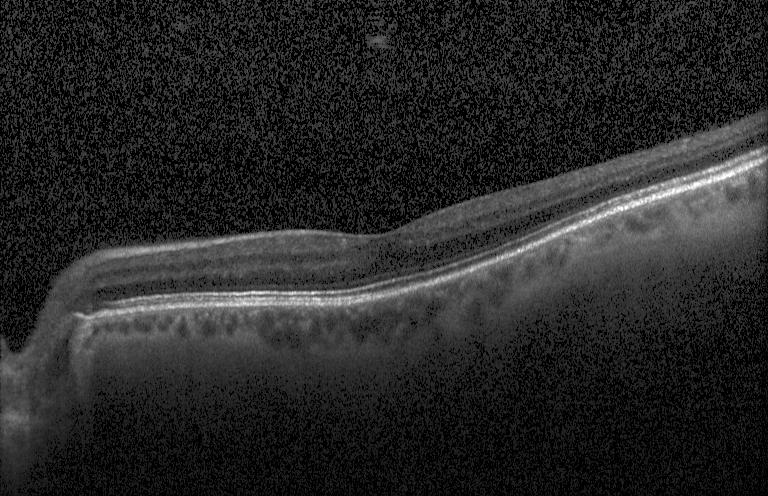 Instrument: Heidelberg Spectralis · optical coherence tomography scan
The scan shows no evidence of choroidal neovascularization, diabetic macular edema, or drusen.